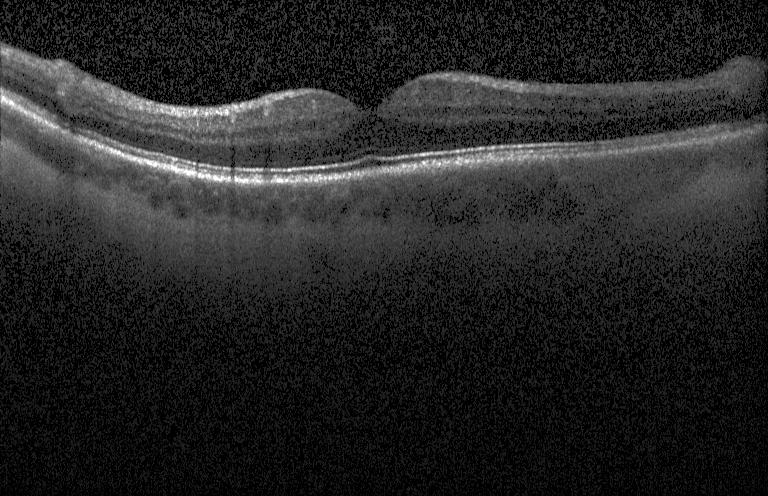 Macular OCT: no CNV, no DME, and no drusen.